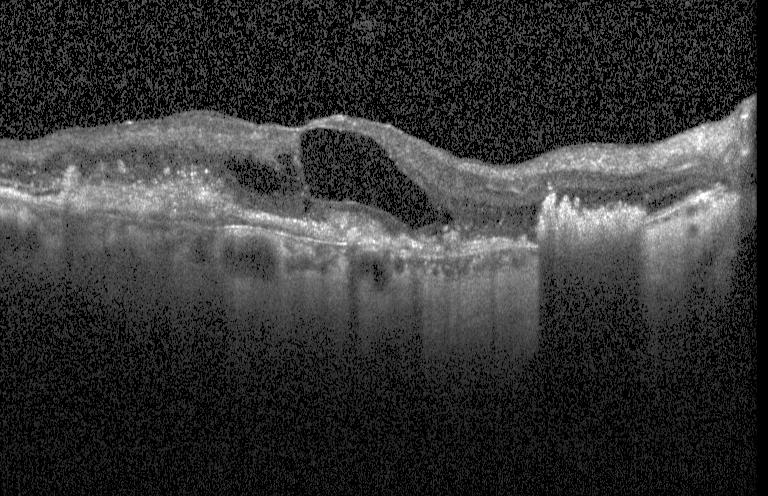
Retinal OCT B-scan. Macular OCT: choroidal neovascularization.